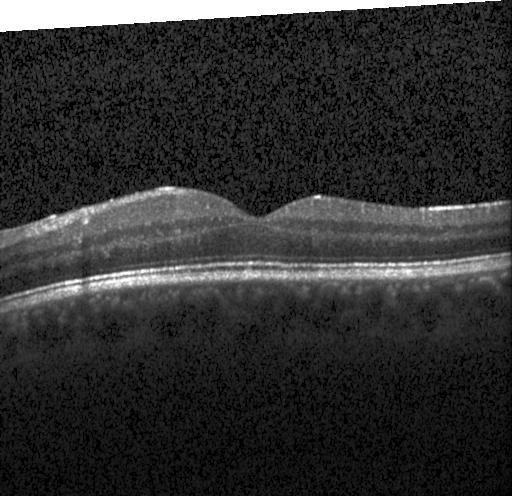
Heidelberg Spectralis; through the macula; OCT line scan; spectral-domain optical coherence tomography
Finding: no CNV, no DME, and no drusen.